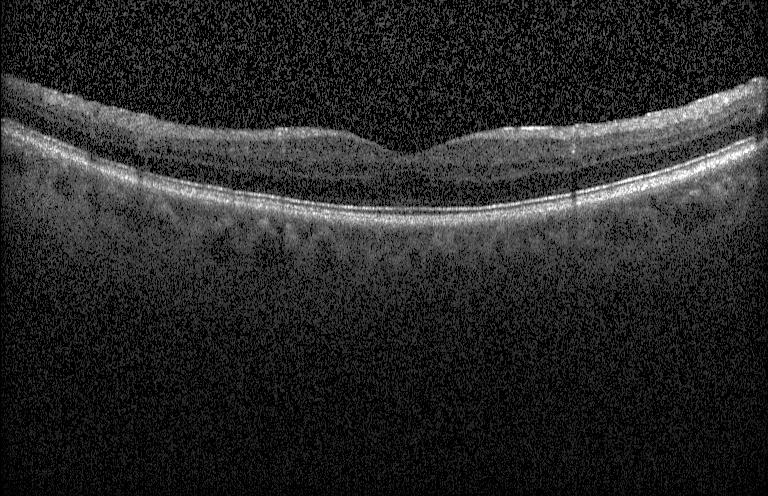 Retinal OCT cross-section showing neither choroidal neovascularization, diabetic macular edema, nor drusen.